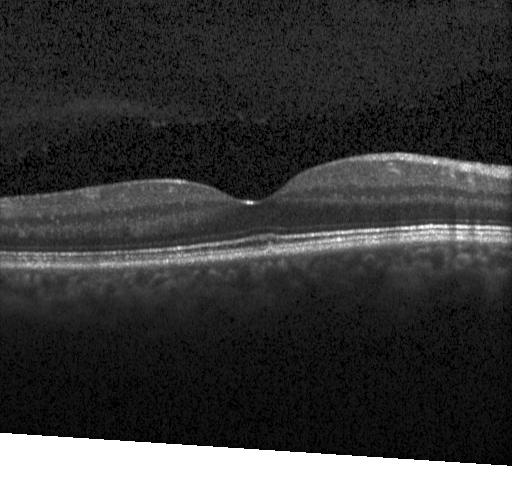 Assessment: no CNV, DME, or drusen.